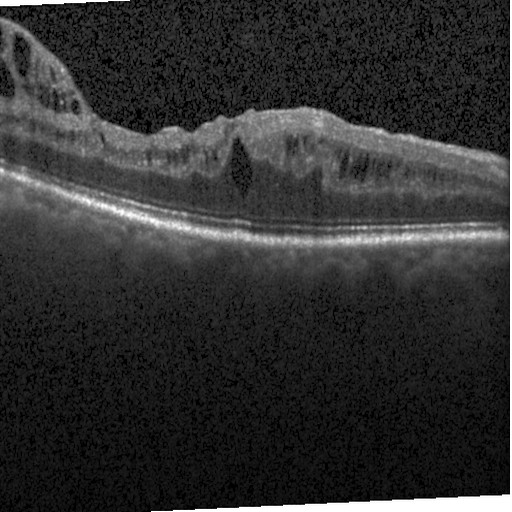 Impression: DME.